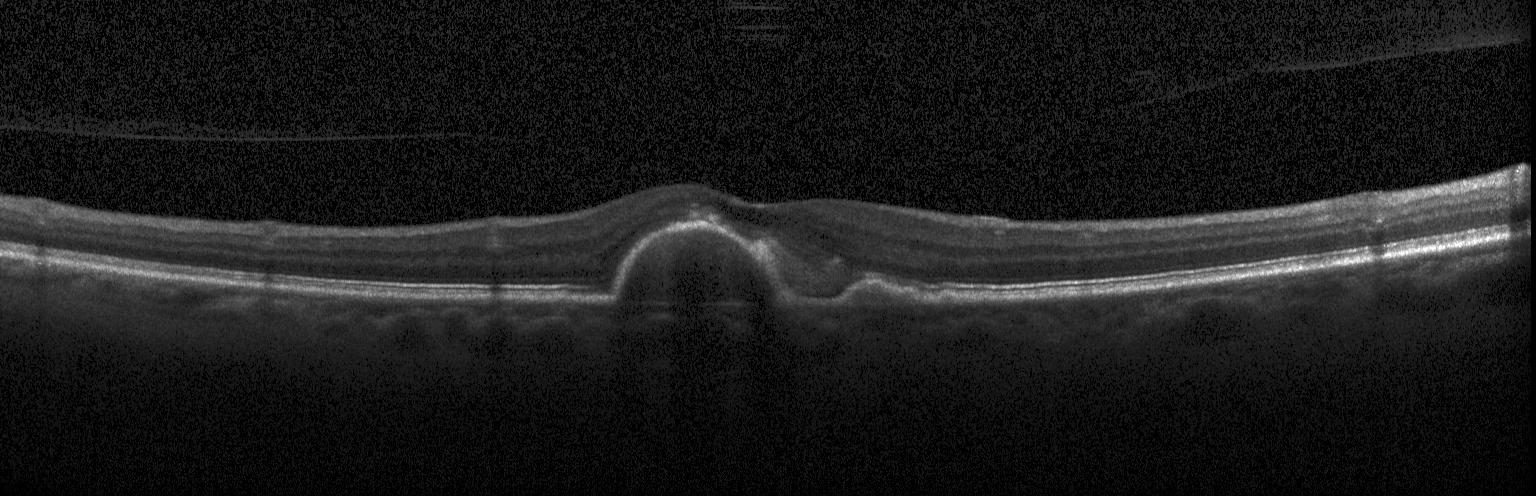
Retinal OCT B-scan · macular scan — This B-scan demonstrates choroidal neovascularization (CNV).